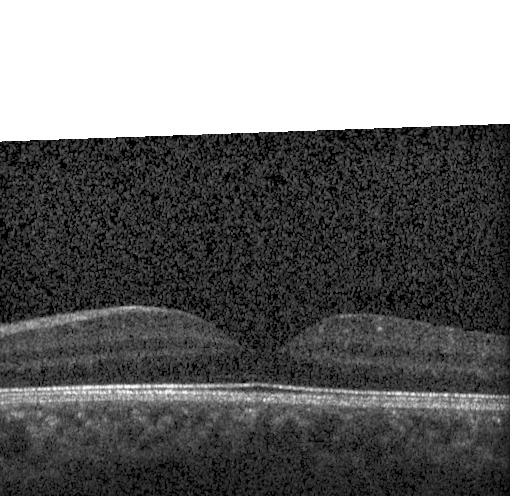 Heidelberg Spectralis, retinal OCT cross-section.
This B-scan demonstrates neither choroidal neovascularization, diabetic macular edema, nor drusen.